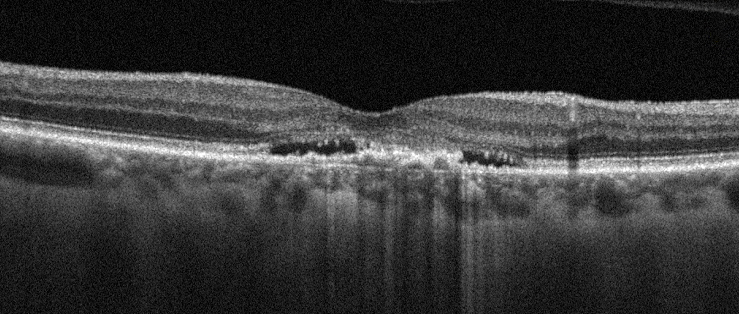

Optical coherence tomography B-scan.
The scan shows AMD.